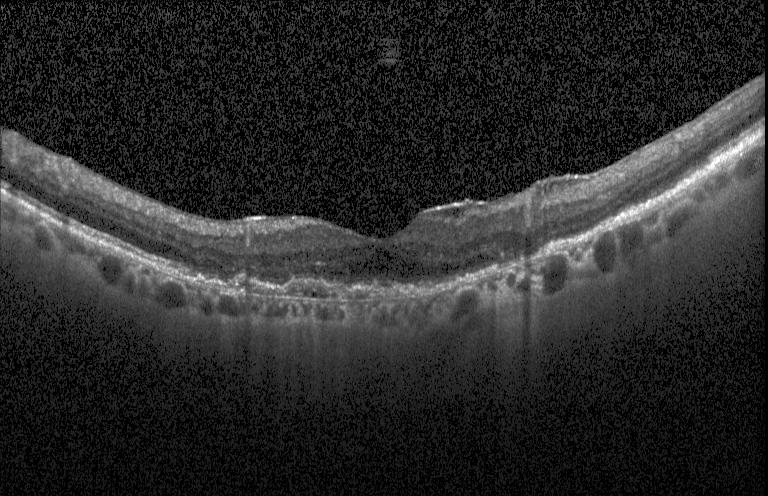 Acquired on a Heidelberg Spectralis. OCT line scan
OCT finding: choroidal neovascularization (CNV).